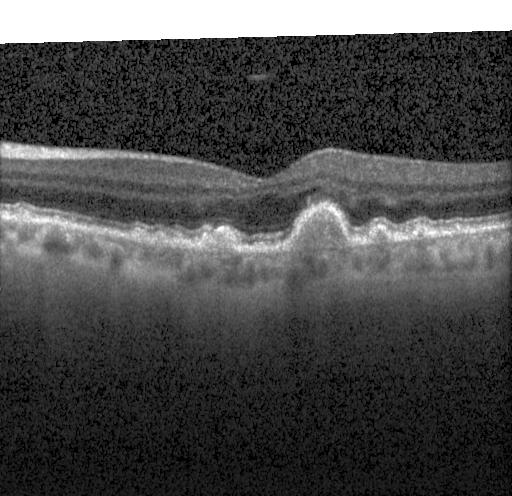

Macular OCT demonstrating sub-RPE drusenoid deposits.